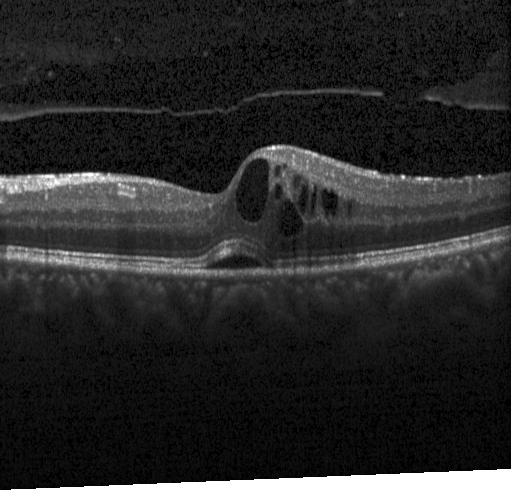 OCT scan showing diabetic macular edema (DME).